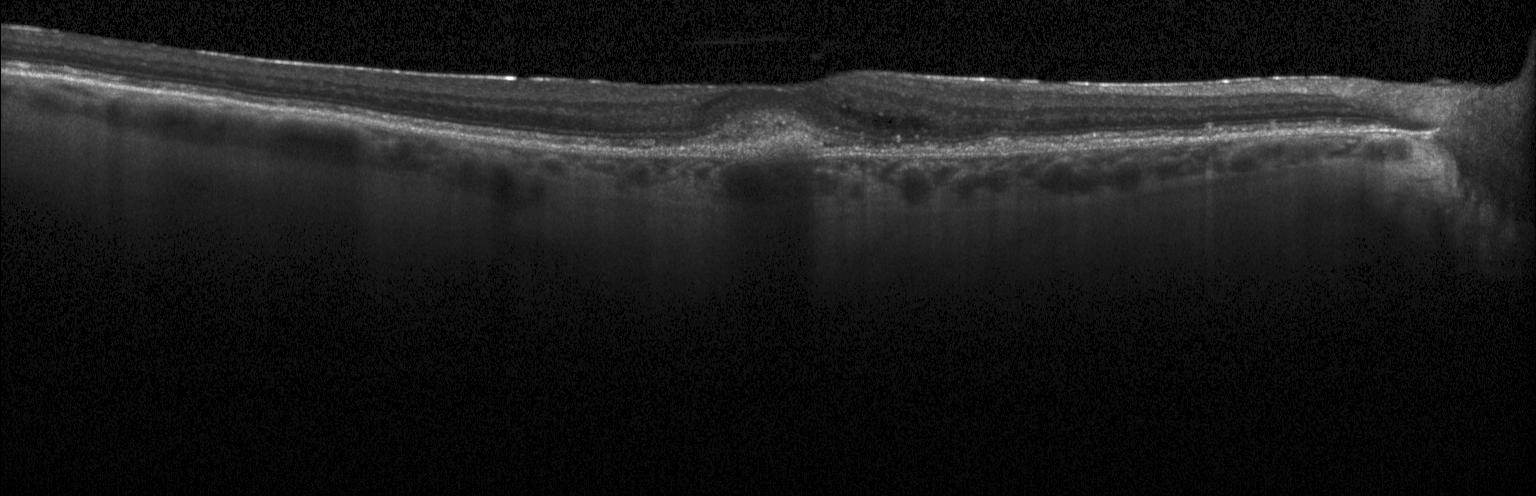

Optical coherence tomography B-scan
This B-scan demonstrates a choroidal neovascular membrane.